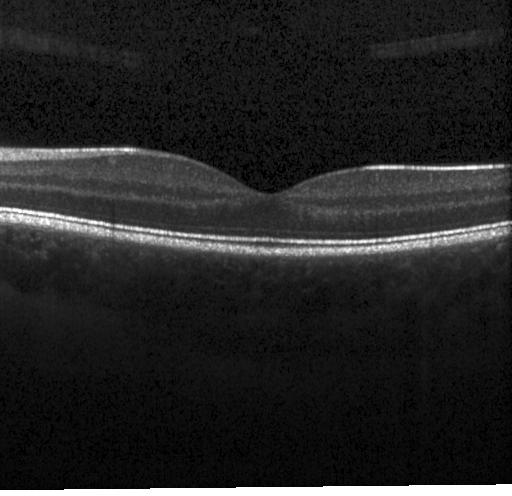

Optical coherence tomography B-scan · instrument: Heidelberg Spectralis — Dx: neither choroidal neovascularization, diabetic macular edema, nor drusen.